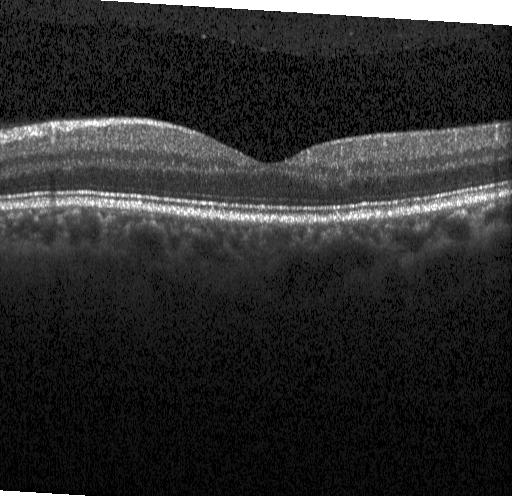

Impression: no evidence of CNV, DME, or drusen.